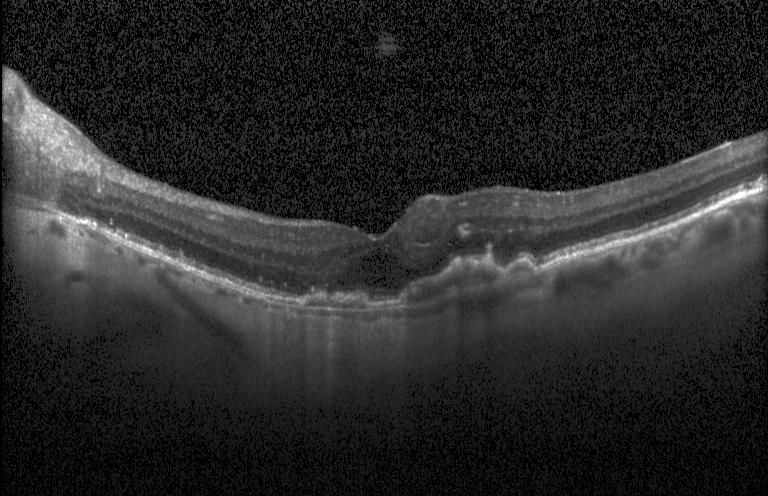
Finding: a choroidal neovascular membrane.